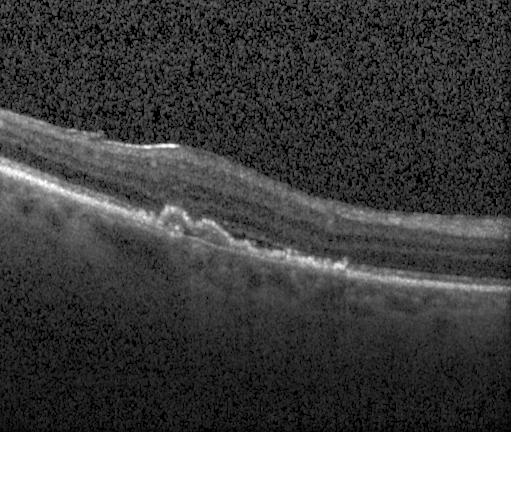

Heidelberg Spectralis OCT system. Optical coherence tomography B-scan. Fovea-centered. SD-OCT.
This B-scan demonstrates a choroidal neovascular membrane.